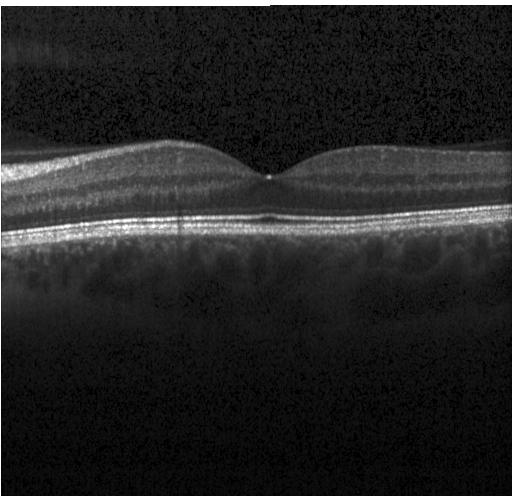
Retinal OCT cross-section showing neither choroidal neovascularization, diabetic macular edema, nor drusen.